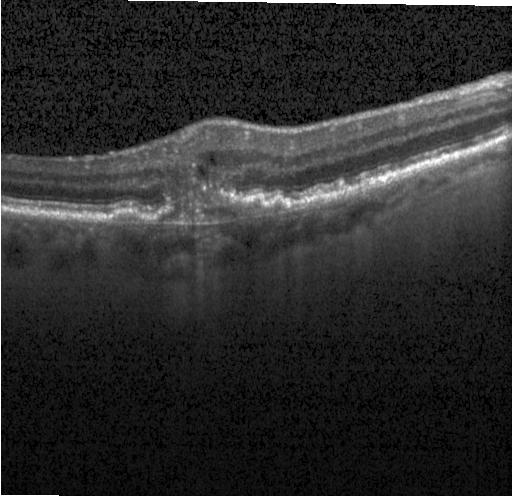
Retinal OCT cross-section. A choroidal neovascular membrane.